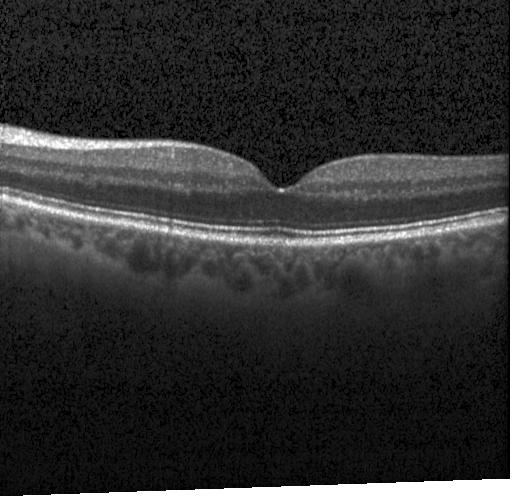 Optical coherence tomography B-scan; SD-OCT
Impression: no evidence of CNV, DME, or drusen.